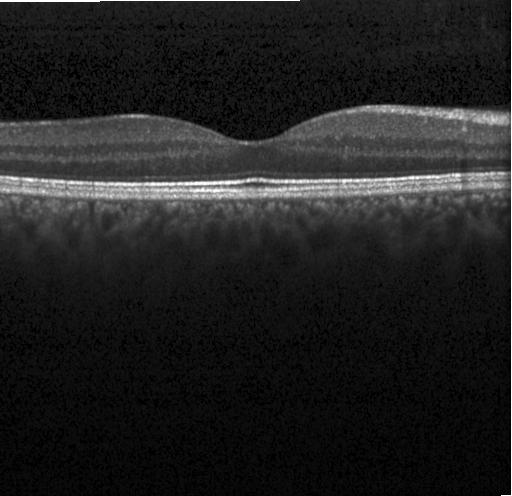
Macular OCT demonstrating no CNV, no DME, and no drusen.